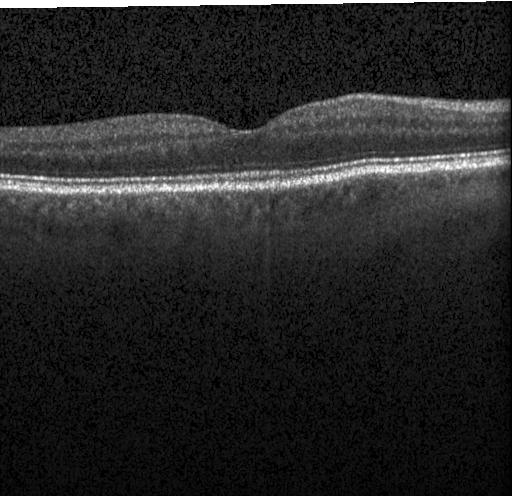 Fovea-centered; spectral-domain optical coherence tomography; OCT line scan; Heidelberg Spectralis.
Finding: no choroidal neovascularization, no diabetic macular edema, and no drusen.